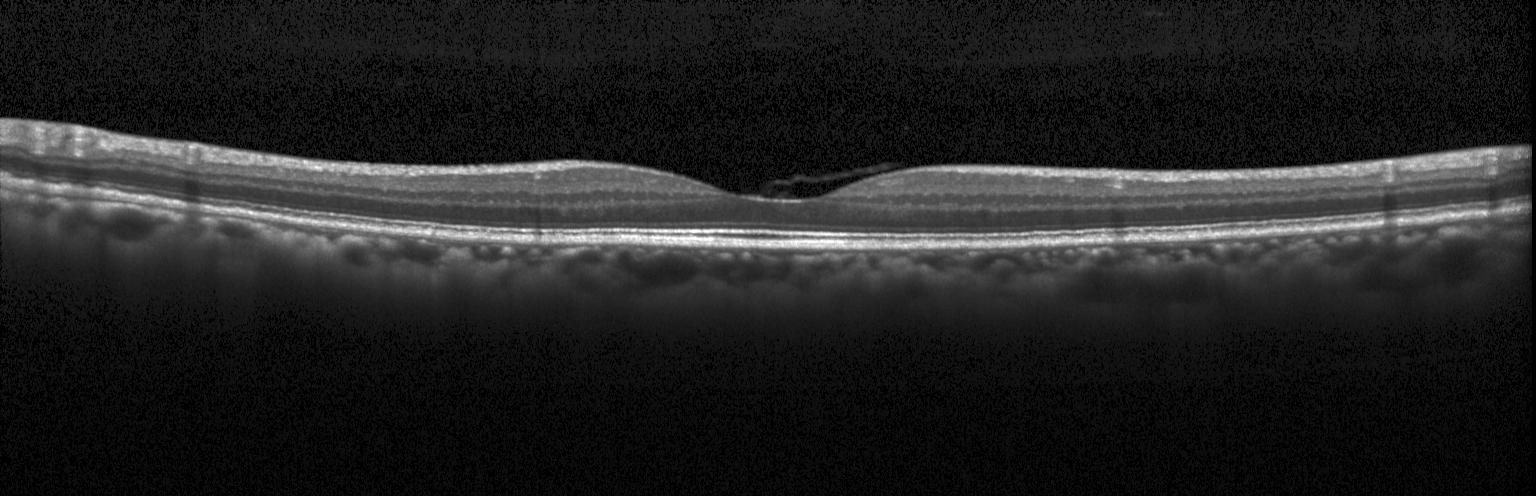
OCT B-scan showing no choroidal neovascularization, diabetic macular edema, or drusen.